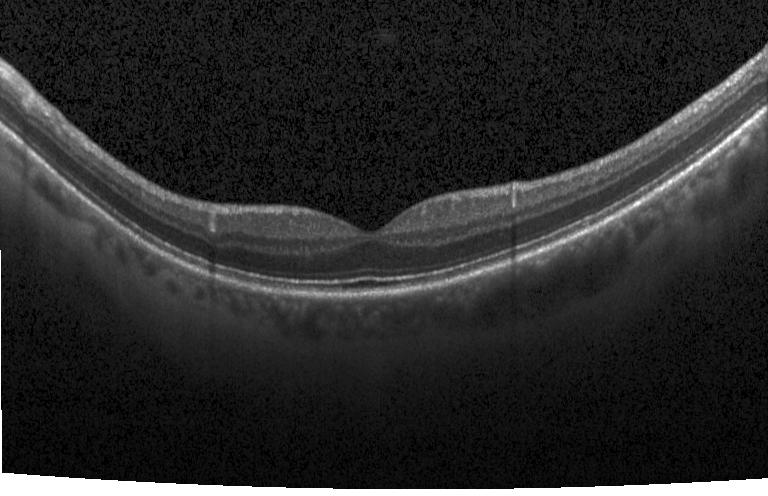

Dx: neither choroidal neovascularization, diabetic macular edema, nor drusen.